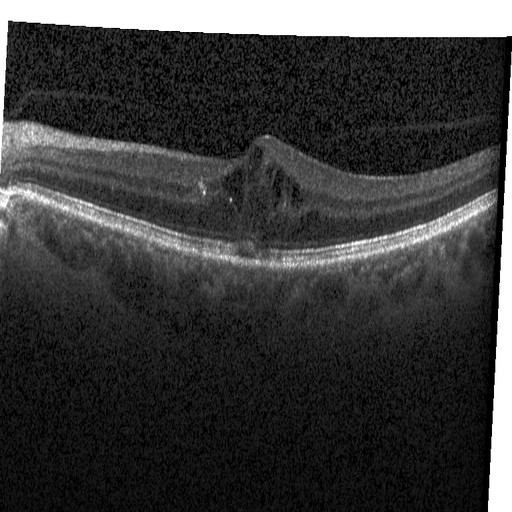

Macular scan. Spectral-domain optical coherence tomography. OCT line scan.
Impression: diabetic macular edema.